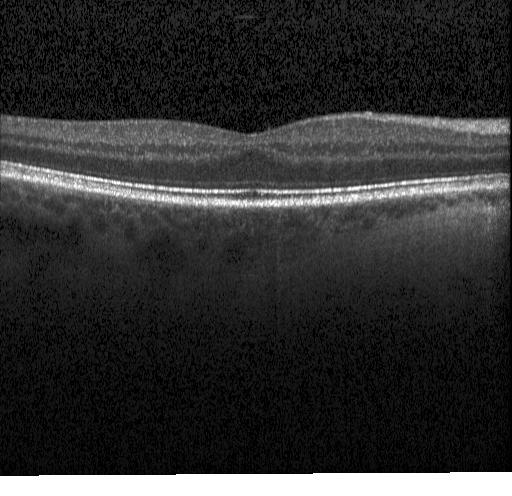 SD-OCT · acquired on a Heidelberg Spectralis · retinal OCT cross-section · centered on the fovea
Finding: neither choroidal neovascularization, diabetic macular edema, nor drusen.